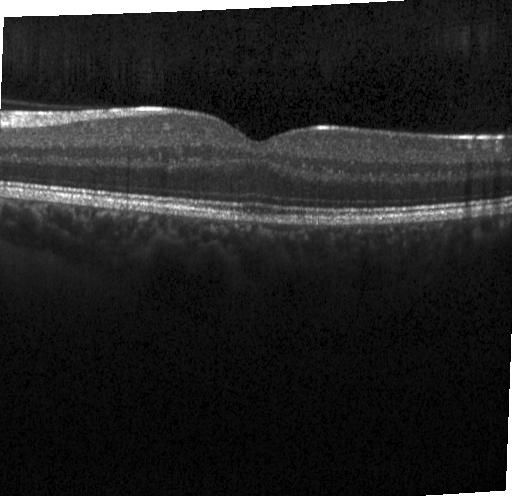
Macular OCT: no evidence of choroidal neovascularization, diabetic macular edema, or drusen.